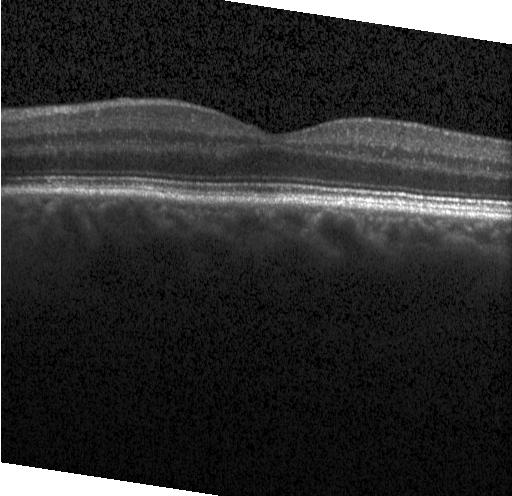 Impression: no CNV, DME, or drusen.